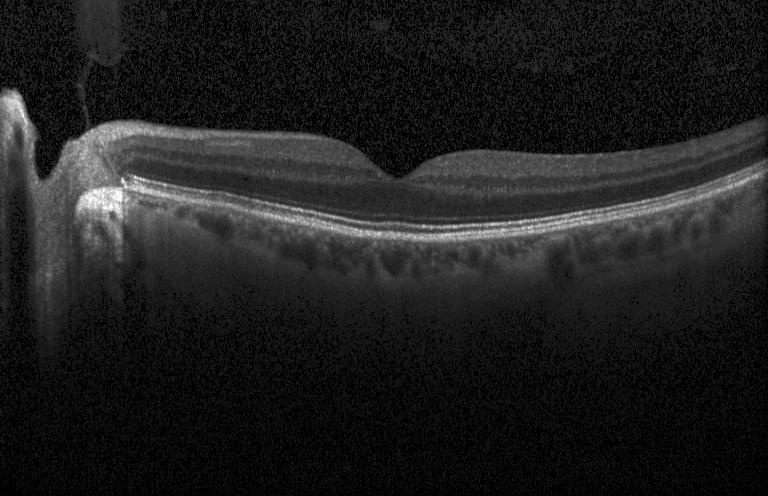

OCT line scan, centered on the fovea, SD-OCT, Heidelberg Spectralis. Macular OCT: no evidence of CNV, DME, or drusen.